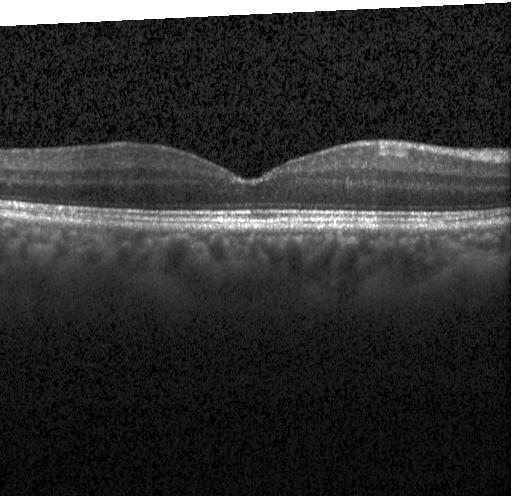
Fovea-centered, retinal OCT cross-section, acquired on a Heidelberg Spectralis.
No evidence of choroidal neovascularization, diabetic macular edema, or drusen.